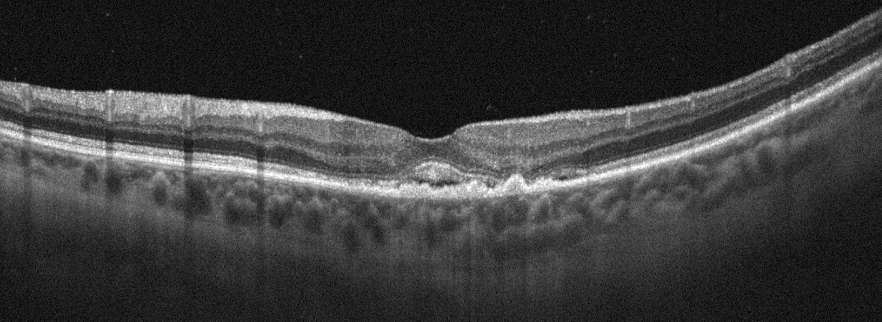

Optical coherence tomography scan, left eye
Diagnosis: AMD.